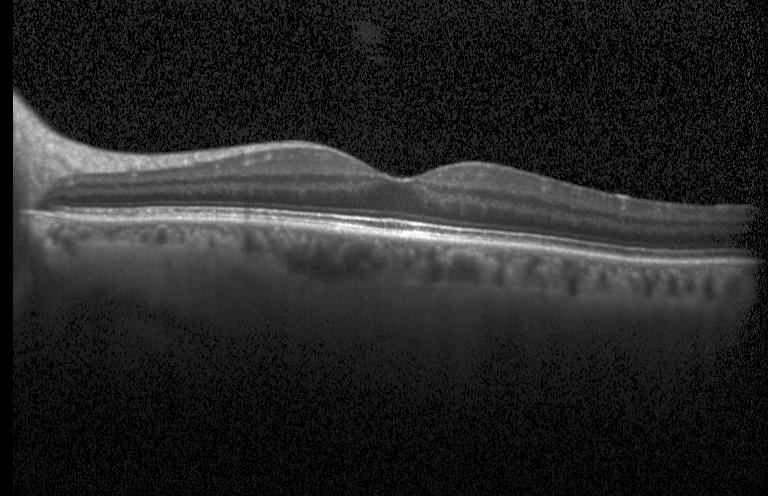 Instrument: Heidelberg Spectralis · retinal OCT B-scan
No choroidal neovascularization, diabetic macular edema, or drusen.